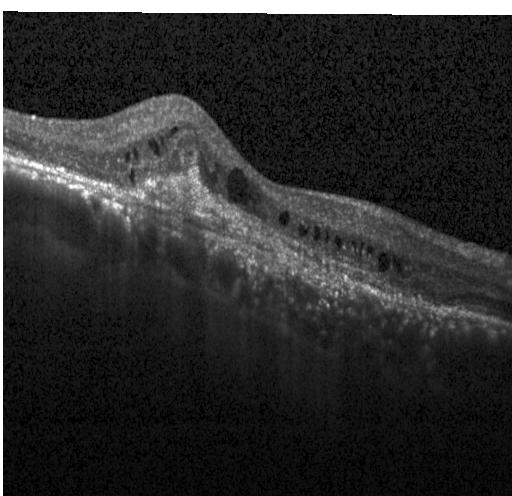
Diagnosis: choroidal neovascularization.